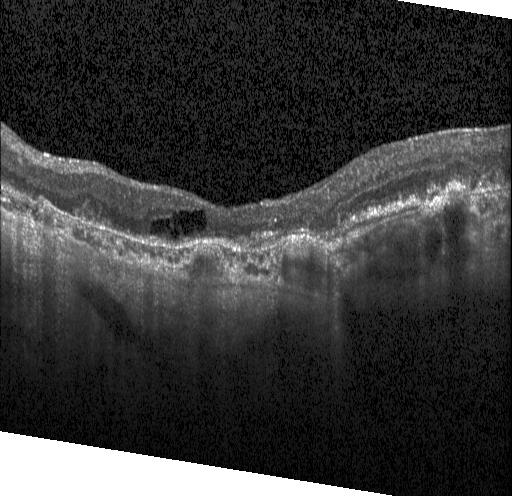 OCT B-scan.
Assessment: a choroidal neovascular membrane.